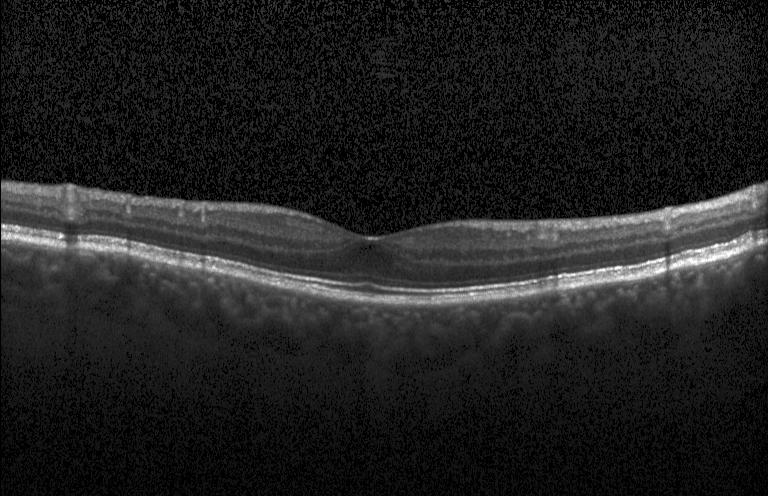
Diagnosis: no CNV, DME, or drusen.